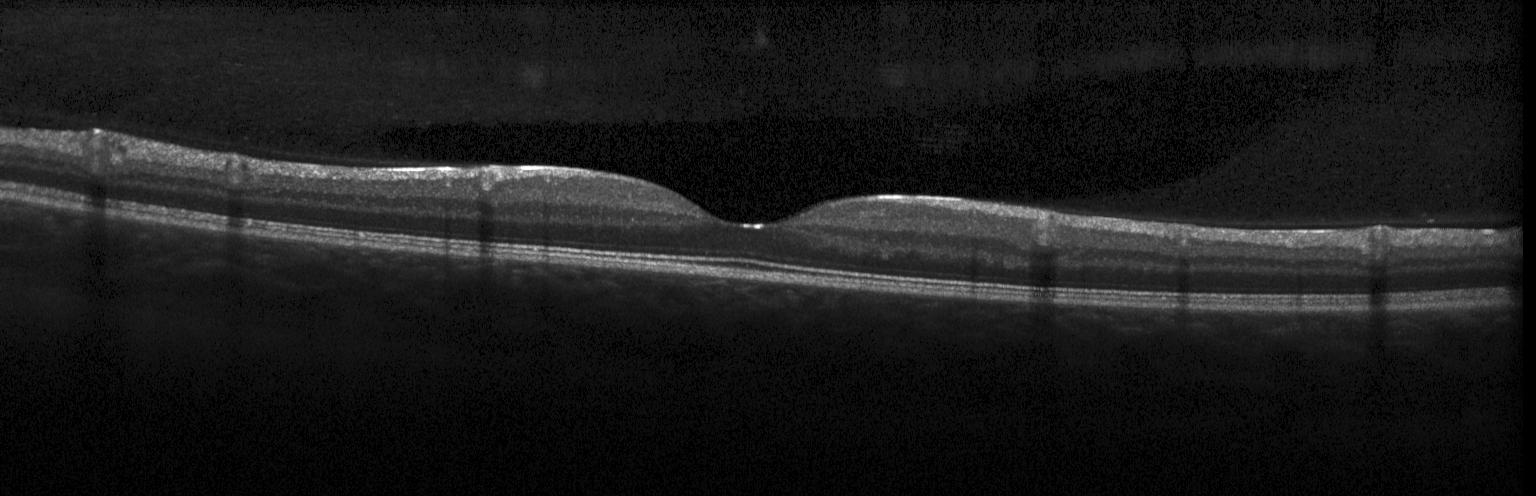 Finding: neither CNV, DME, nor drusen.